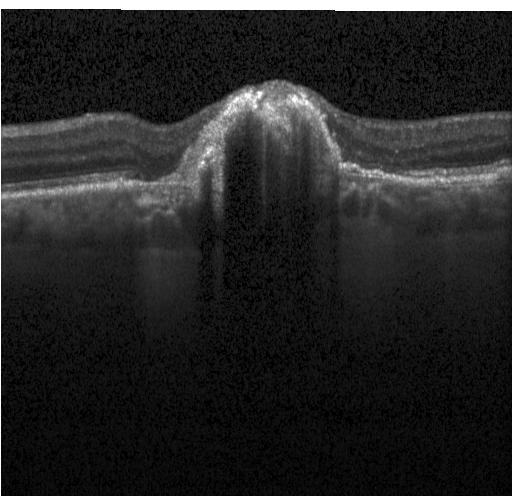

SD-OCT · macular scan · optical coherence tomography scan — This B-scan demonstrates CNV.